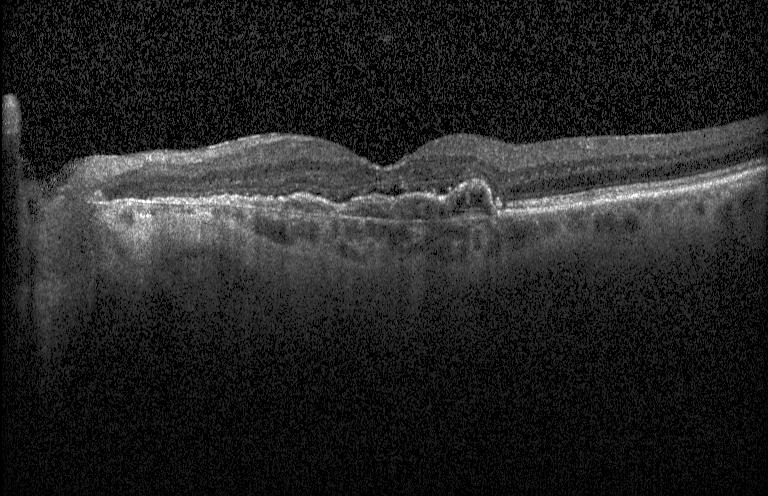 OCT B-scan.
OCT finding: a choroidal neovascular membrane.